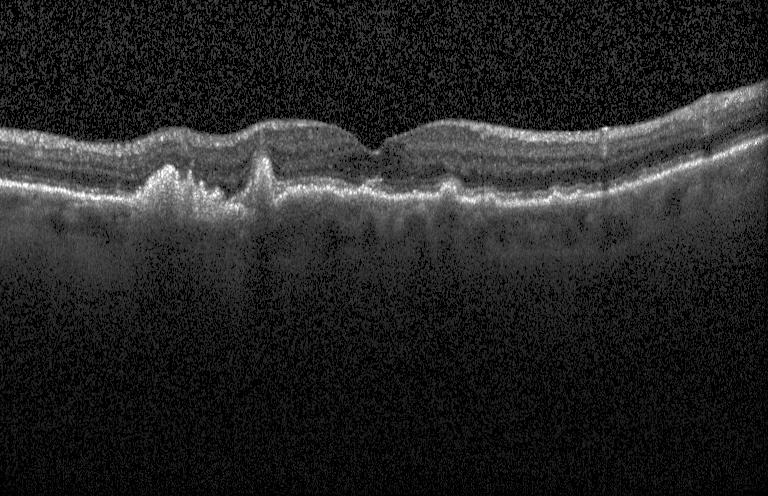 SD-OCT; OCT B-scan; instrument: Heidelberg Spectralis; through the macula. This B-scan demonstrates choroidal neovascularization.